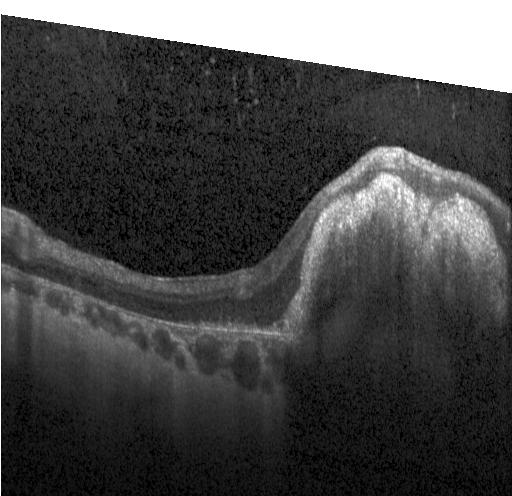 Retinal OCT cross-section
Diagnosis: a choroidal neovascular membrane.